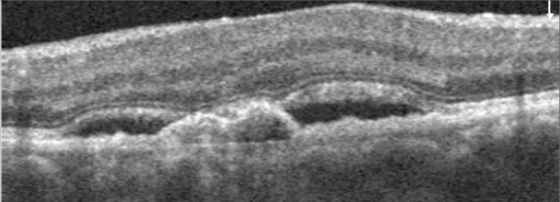

Diagnosis: age-related macular degeneration (AMD).